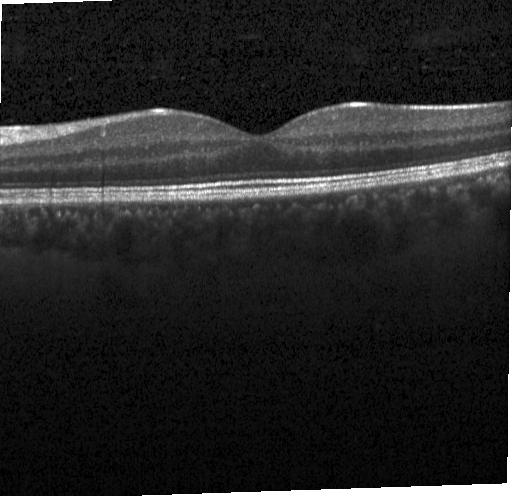

Dx: no choroidal neovascularization, no diabetic macular edema, and no drusen.